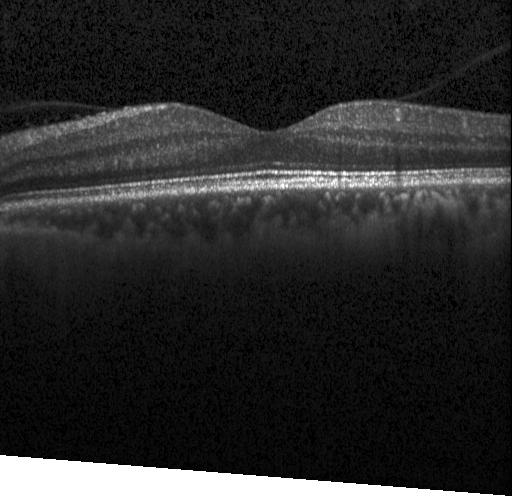
OCT line scan · SD-OCT. Dx: no evidence of choroidal neovascularization, diabetic macular edema, or drusen.